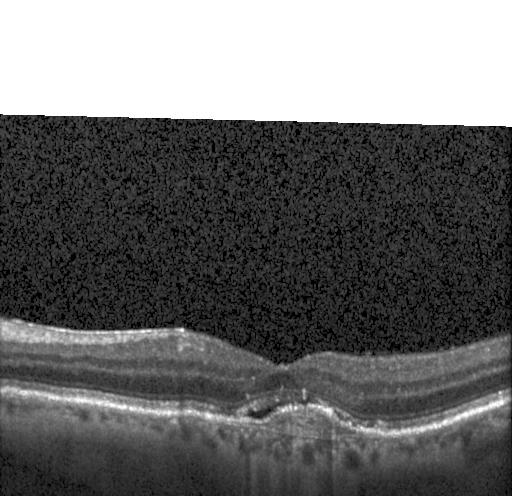

Horizontal scan through the fovea · OCT line scan. Diagnosis: choroidal neovascularization (CNV).